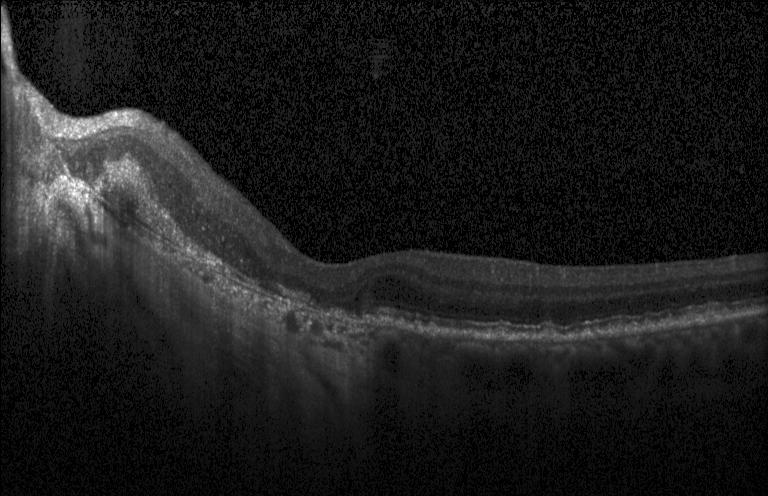

Optical coherence tomography B-scan · spectral-domain OCT.
The scan shows choroidal neovascularization.